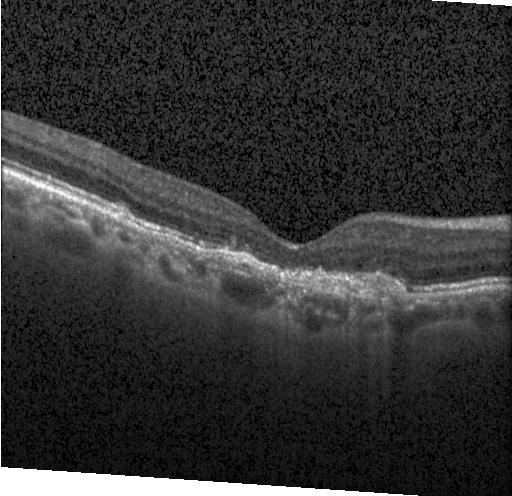

Retinal OCT cross-section; spectral-domain OCT; macular scan
Finding: choroidal neovascularization.